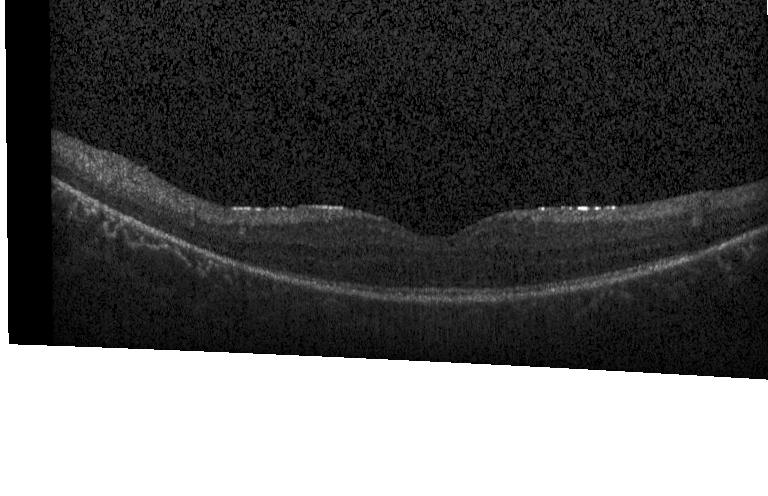
Retinal OCT B-scan · acquired on a Heidelberg Spectralis · spectral-domain optical coherence tomography — OCT finding: neither choroidal neovascularization, diabetic macular edema, nor drusen.